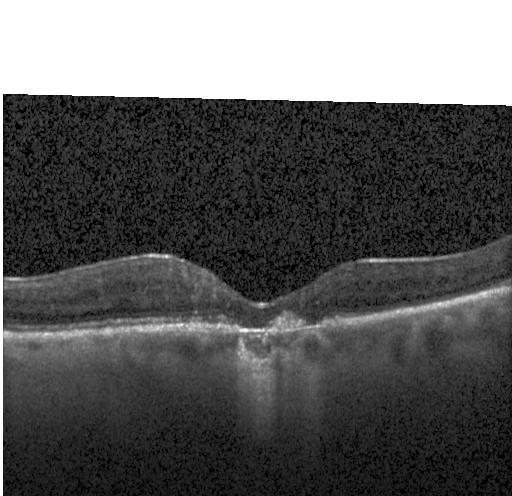
OCT scan showing choroidal neovascularization (CNV).